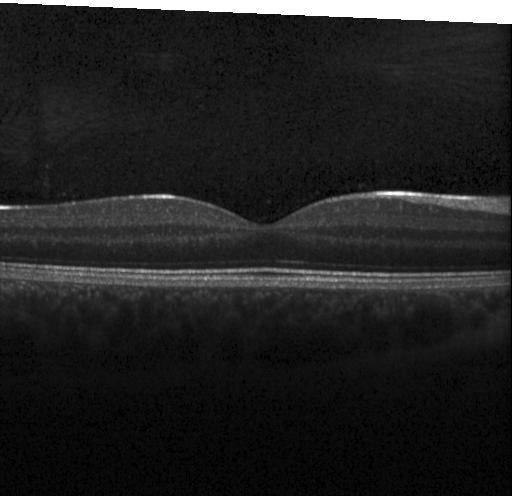 Dx: no CNV, no DME, and no drusen.